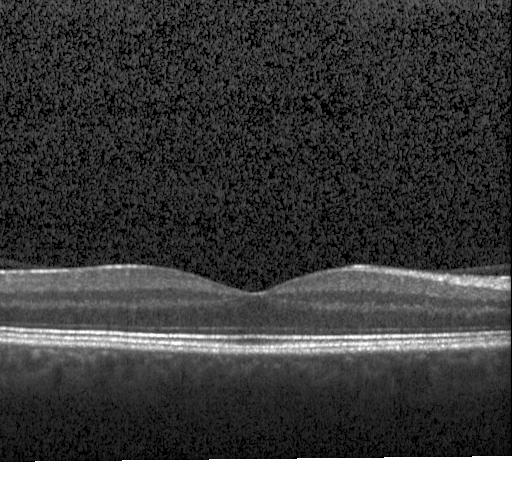 Optical coherence tomography scan — Diagnosis: no choroidal neovascularization, no diabetic macular edema, and no drusen.